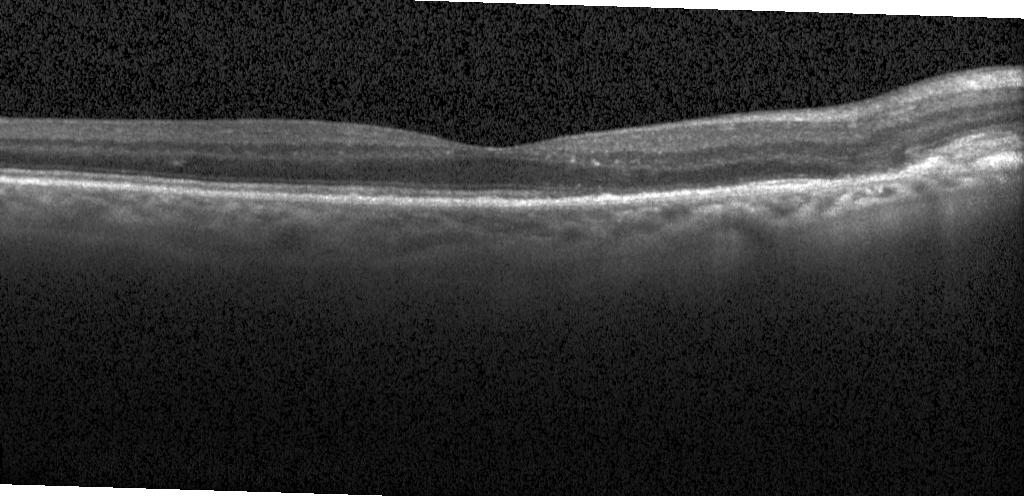

Spectral-domain OCT B-scan: a choroidal neovascular membrane.